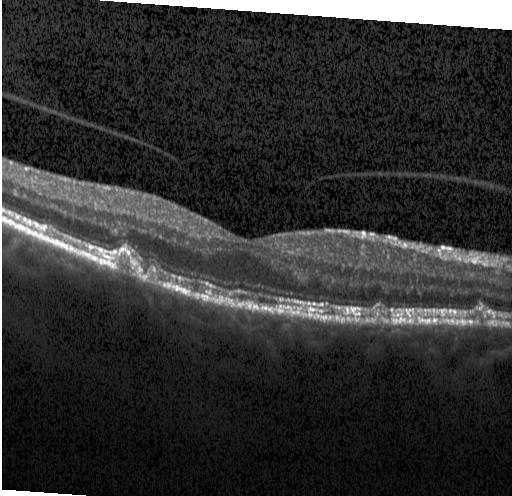

Retinal OCT cross-section showing drusen.